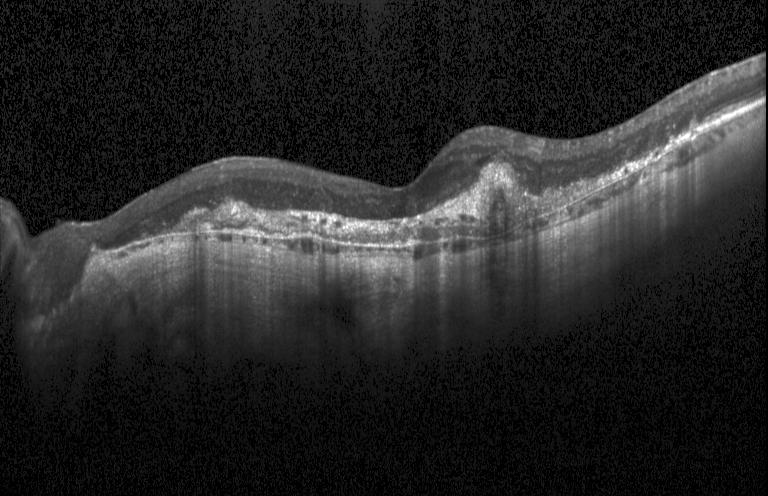

This B-scan demonstrates a choroidal neovascular membrane.